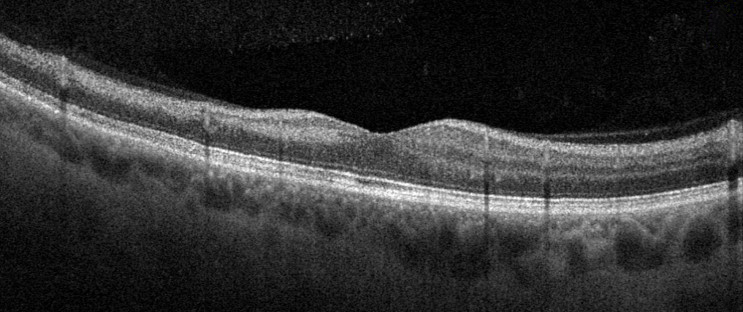

Through the macula; OCT B-scan; acquired on an Optovue Avanti RTVue XR. Dx: RVO.